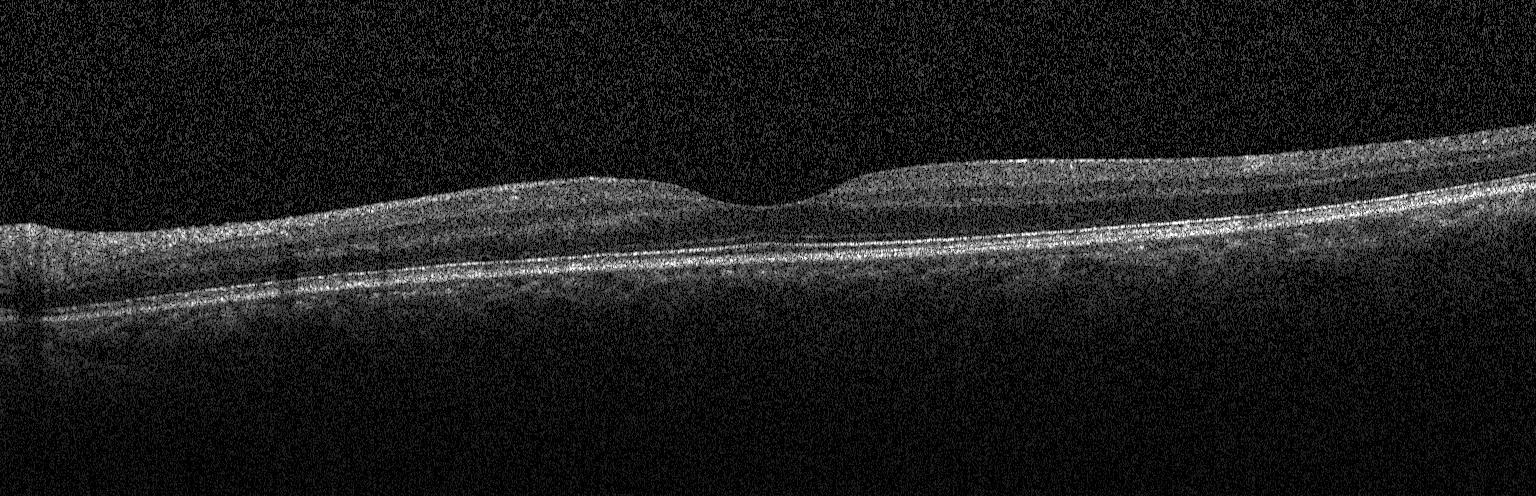
Assessment: neither CNV, DME, nor drusen.